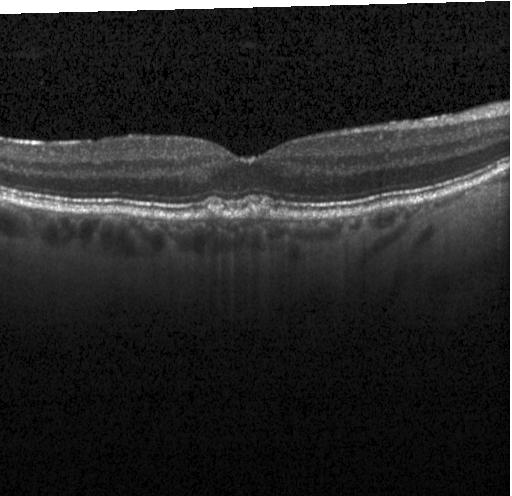
Retinal OCT cross-section. Impression: multiple drusen.